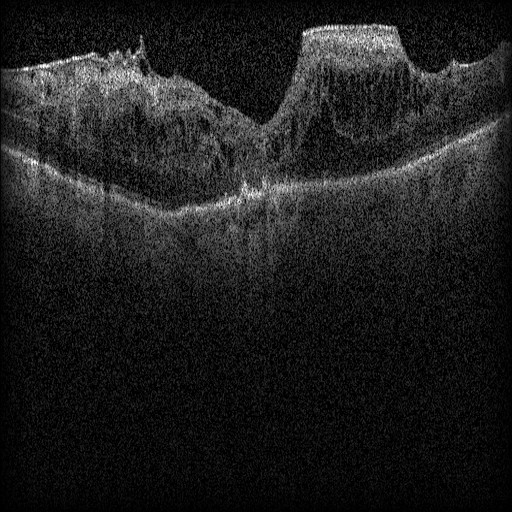

Retinal OCT B-scan · macular scan — Diagnosis: diabetic macular edema (DME).